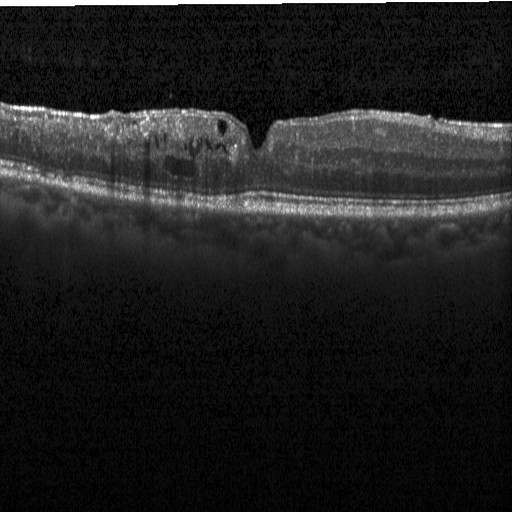

Through the macula; OCT B-scan.
The scan shows diabetic macular edema (DME).